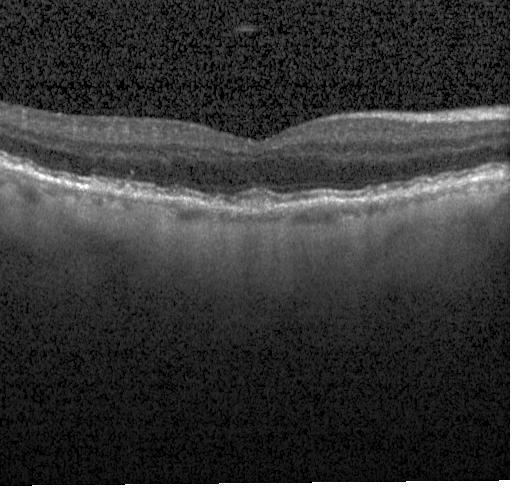 Impression: drusen.